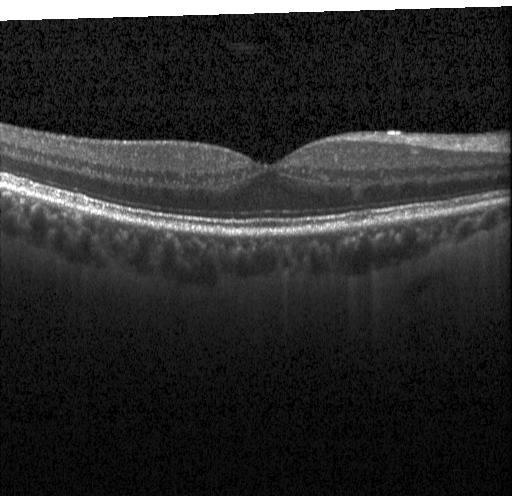

Retinal OCT cross-section — Macular OCT: no CNV, DME, or drusen.